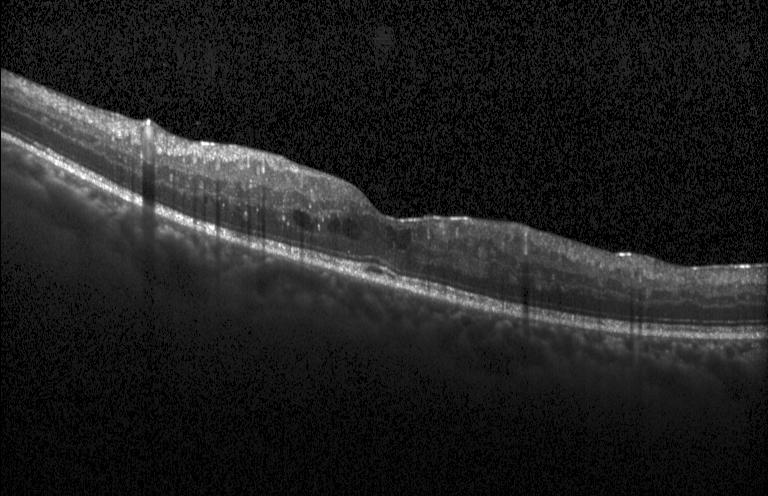
OCT finding: DME.